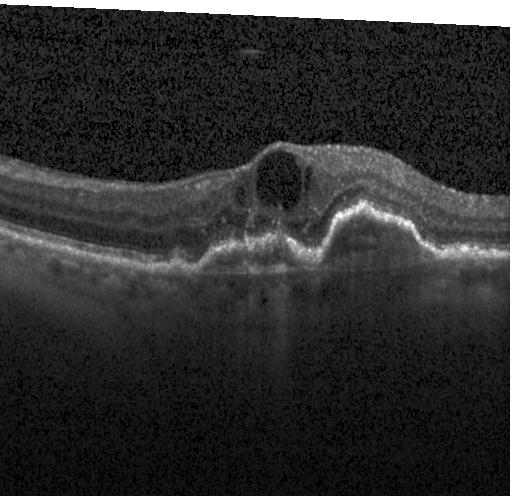
OCT B-scan showing choroidal neovascularization.